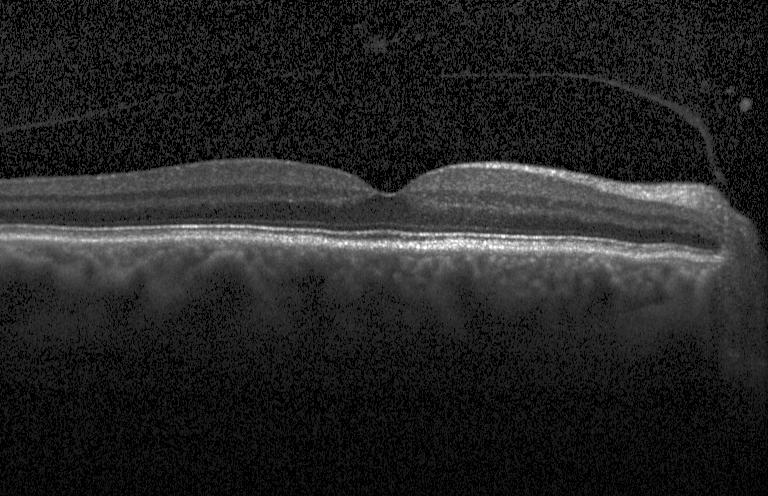

Finding: no choroidal neovascularization, no diabetic macular edema, and no drusen.